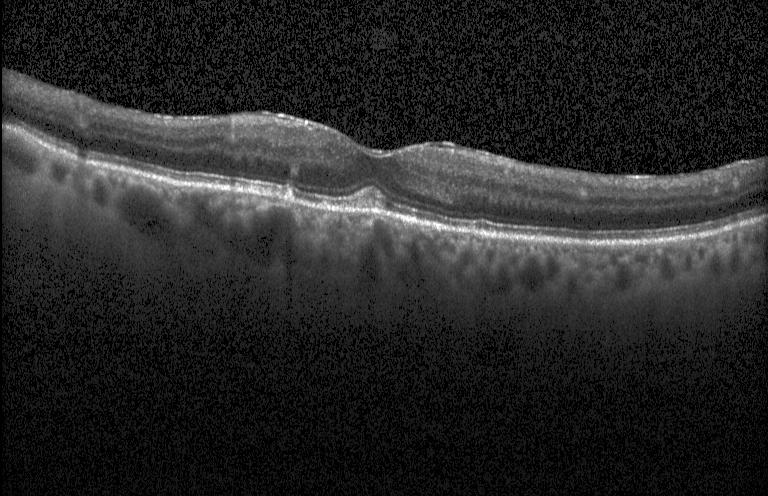

Diagnosis: multiple drusen.